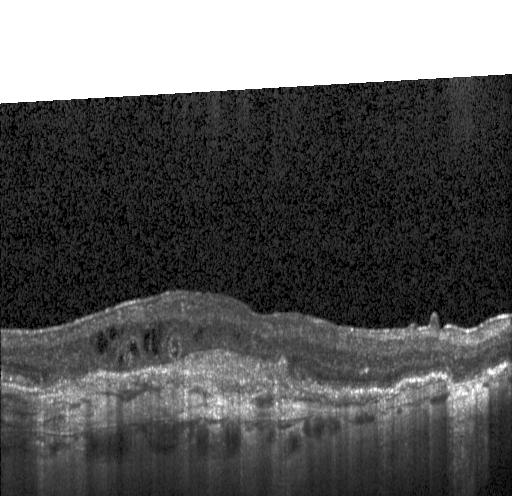
Retinal OCT B-scan. Impression: CNV.